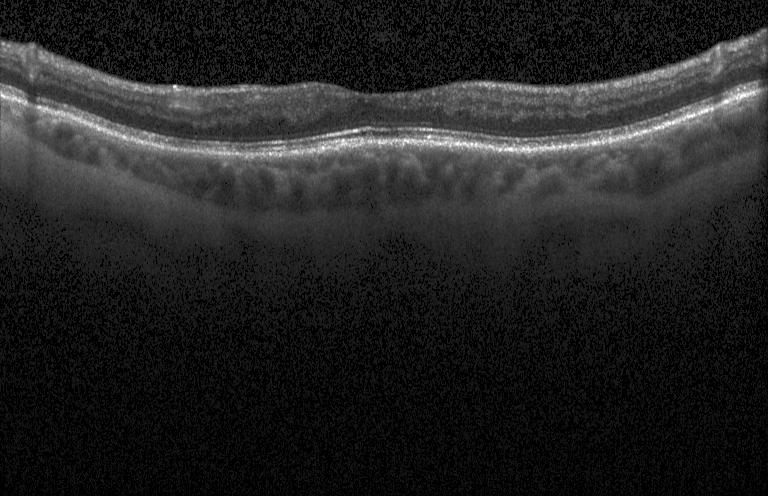

OCT B-scan — The scan shows no evidence of choroidal neovascularization, diabetic macular edema, or drusen.